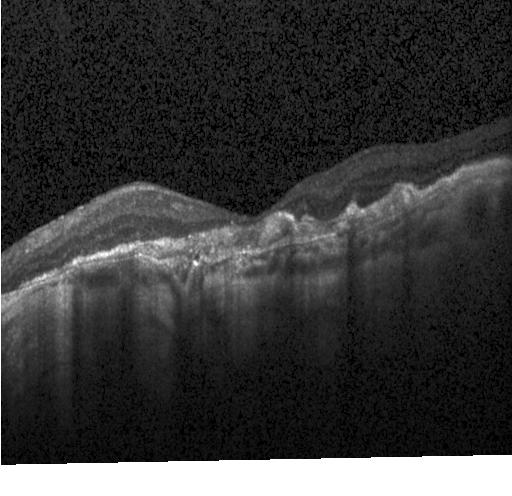

OCT scan showing a choroidal neovascular membrane.